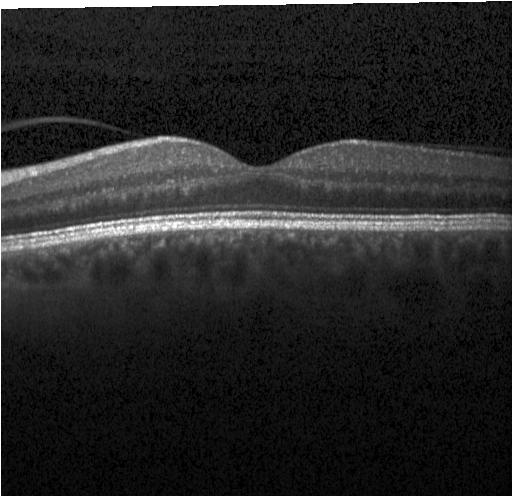
OCT line scan, spectral-domain OCT. Finding: no evidence of CNV, DME, or drusen.